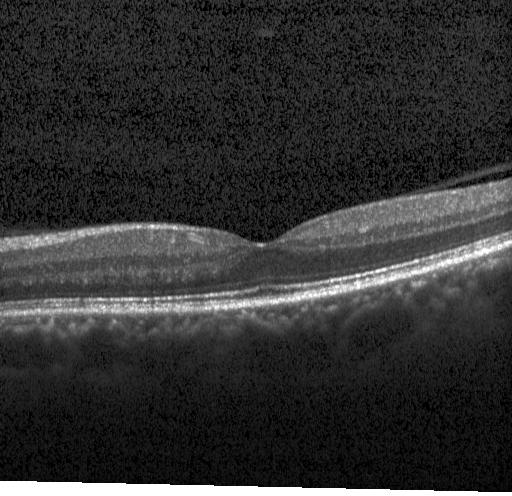

Retinal OCT cross-section.
No choroidal neovascularization, no diabetic macular edema, and no drusen.